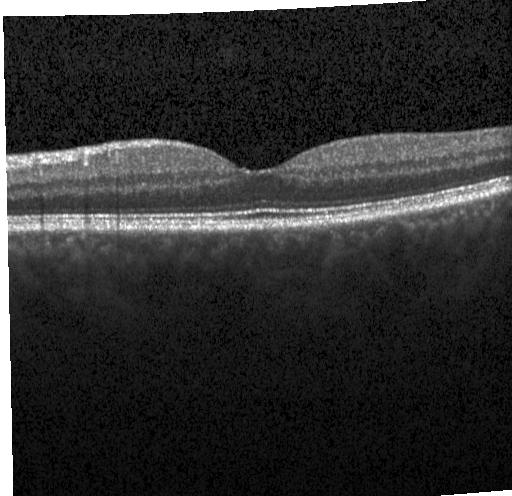 Optical coherence tomography scan · Heidelberg Spectralis. Impression: no choroidal neovascularization, diabetic macular edema, or drusen.